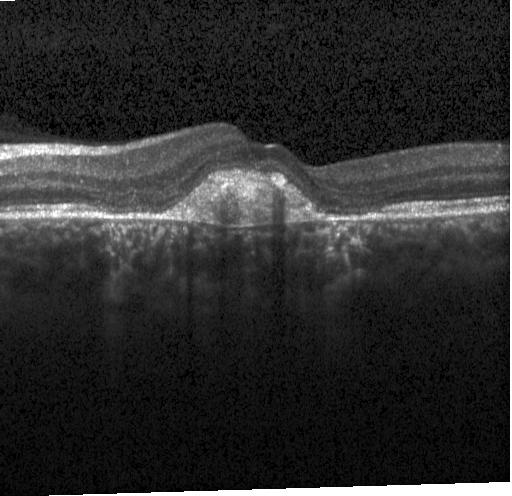
SD-OCT · macular scan · OCT B-scan · acquired on a Heidelberg Spectralis.
Diagnosis: a choroidal neovascular membrane.